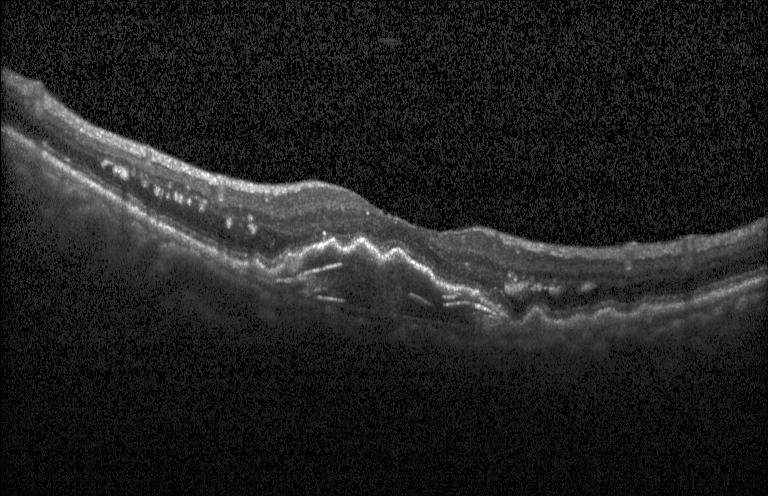
OCT B-scan showing choroidal neovascularization (CNV).